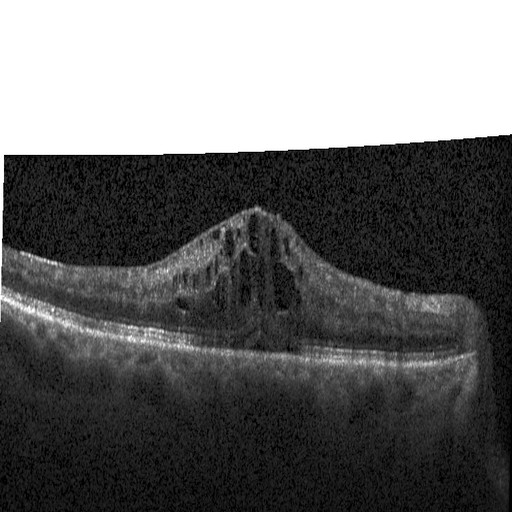 OCT line scan. Fovea-centered.
Assessment: DME.